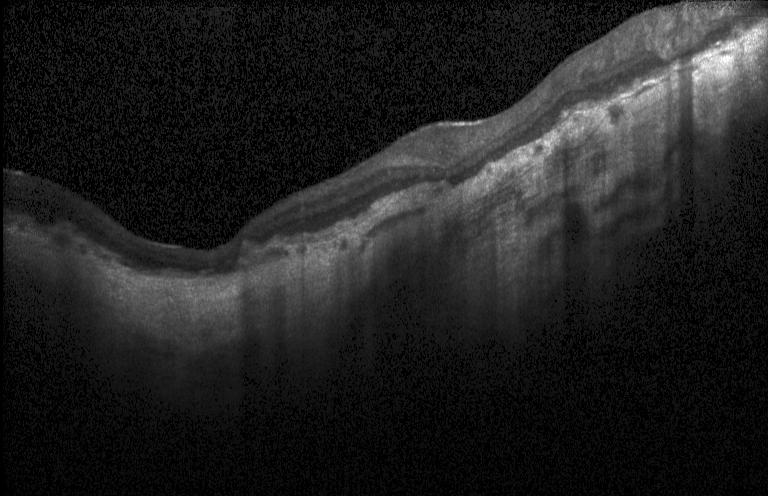 Spectral-domain OCT B-scan: choroidal neovascularization (CNV).